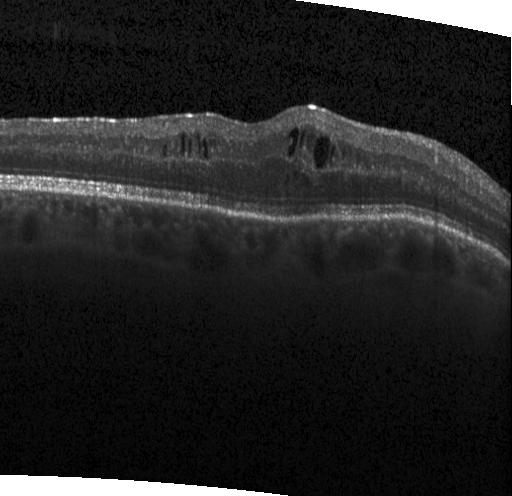

Optical coherence tomography B-scan · Heidelberg Spectralis · SD-OCT
Assessment: diabetic macular edema (DME).